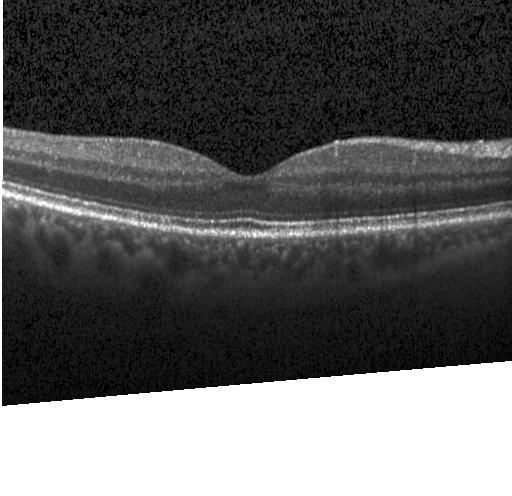
Spectral-domain OCT · acquired on a Heidelberg Spectralis · OCT line scan.
OCT finding: no CNV, DME, or drusen.